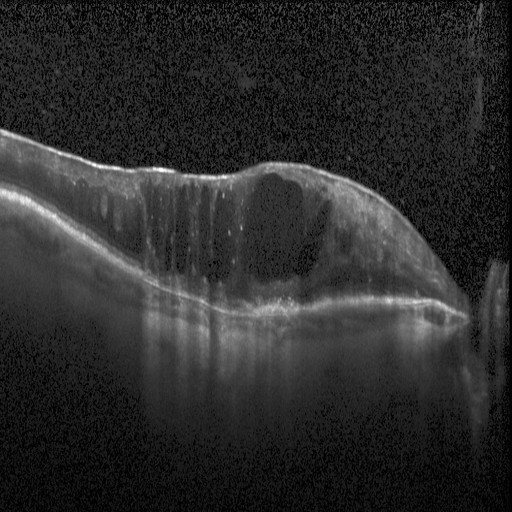

Fovea-centered. Retinal OCT B-scan. SD-OCT. Heidelberg Spectralis
Assessment: diabetic macular edema.